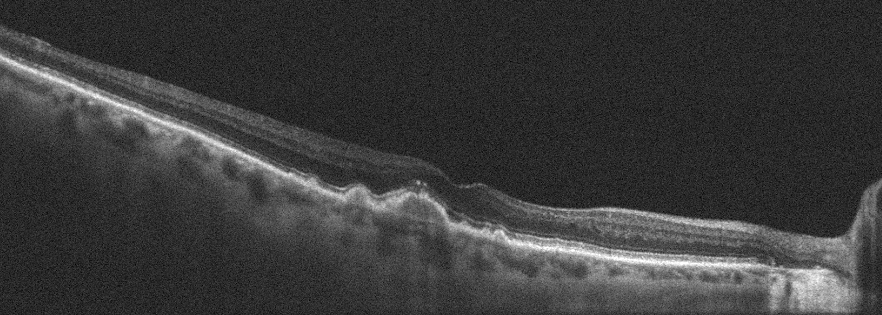

Optical coherence tomography B-scan · oculus dexter · Optovue Avanti RTVue XR.
Finding: age-related macular degeneration (AMD).